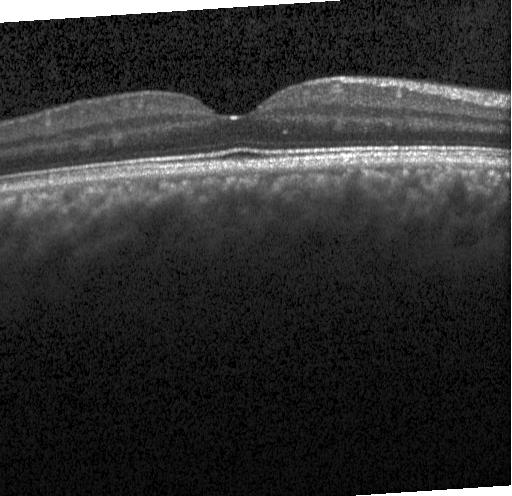 Through the macula · OCT B-scan · Heidelberg Spectralis — No CNV, no DME, and no drusen.